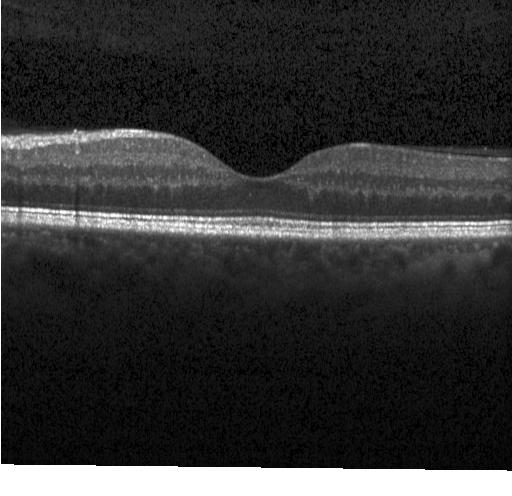 Retinal OCT cross-section. Acquired on a Heidelberg Spectralis. Assessment: no CNV, DME, or drusen.